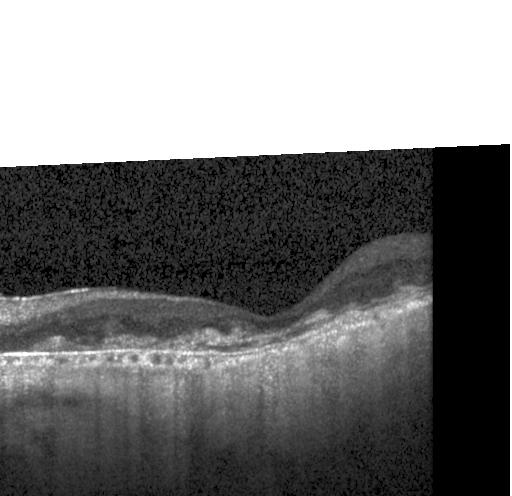

The scan shows a choroidal neovascular membrane.